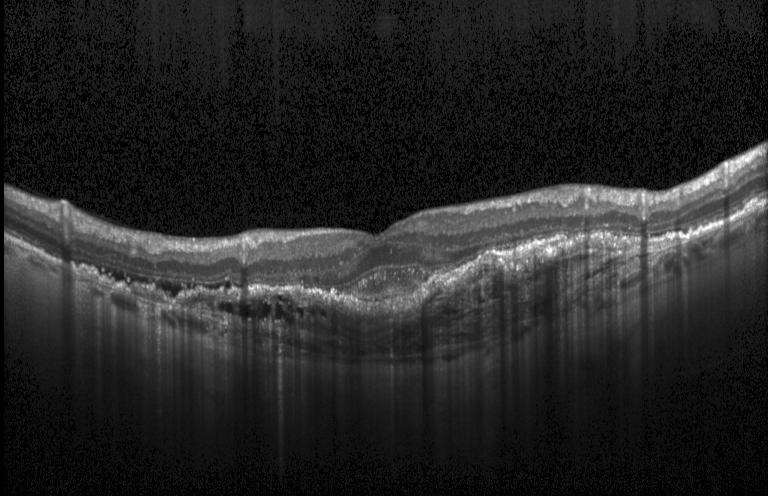
Spectral-domain OCT · retinal OCT B-scan · instrument: Heidelberg Spectralis — OCT finding: a choroidal neovascular membrane.